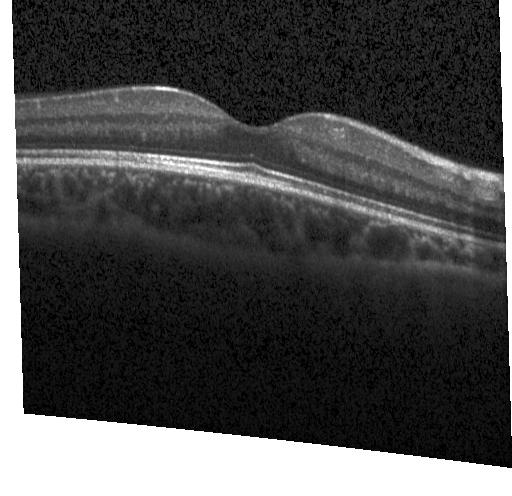

Finding: no evidence of choroidal neovascularization, diabetic macular edema, or drusen.